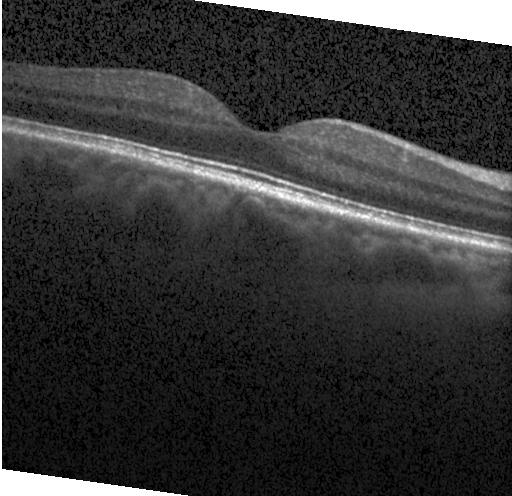
Acquired on a Heidelberg Spectralis, fovea-centered, OCT B-scan, spectral-domain OCT.
Diagnosis: no evidence of choroidal neovascularization, diabetic macular edema, or drusen.